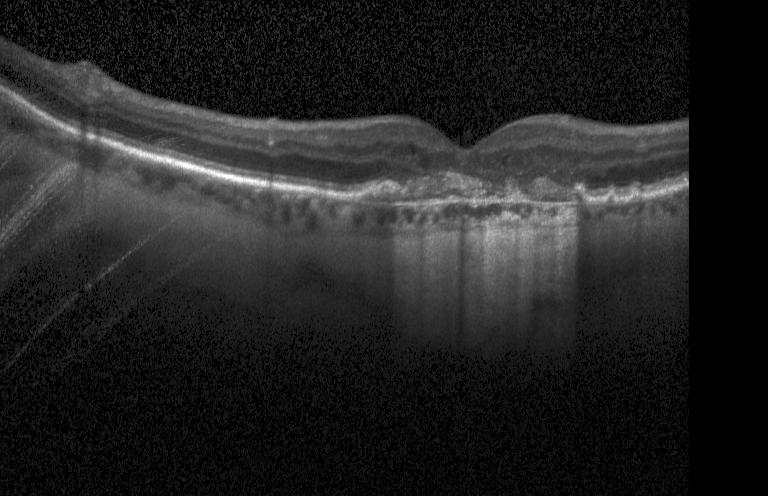
OCT B-scan.
The scan shows a choroidal neovascular membrane.